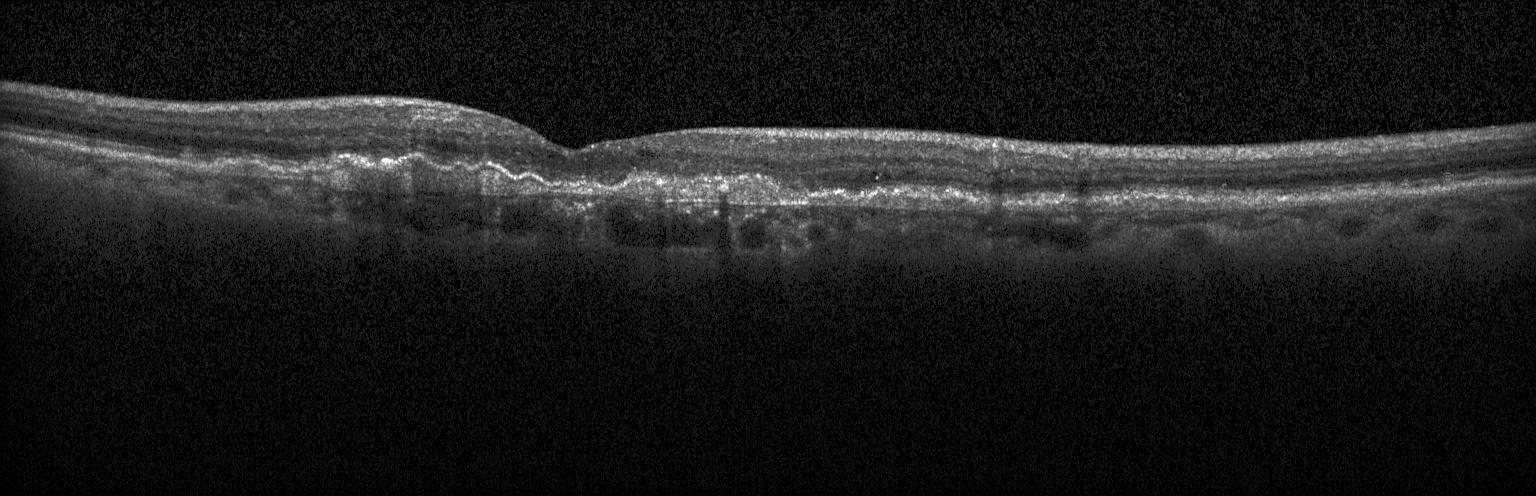
Retinal OCT cross-section. Spectral-domain OCT. Choroidal neovascularization.